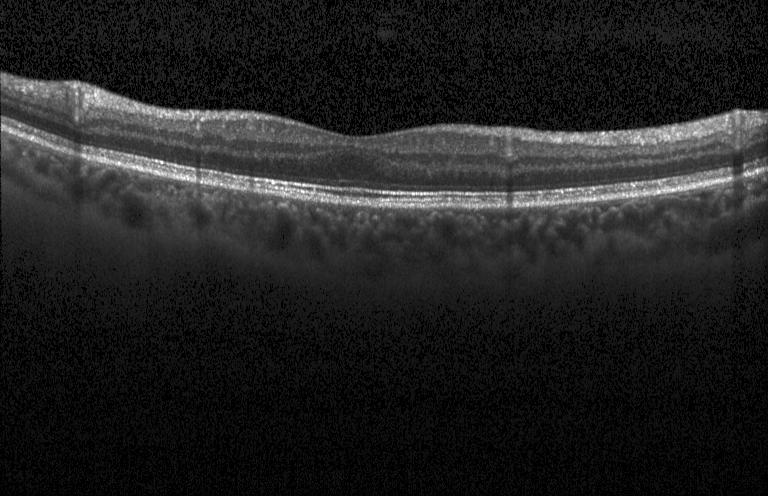
Optical coherence tomography B-scan.
This B-scan demonstrates no CNV, no DME, and no drusen.